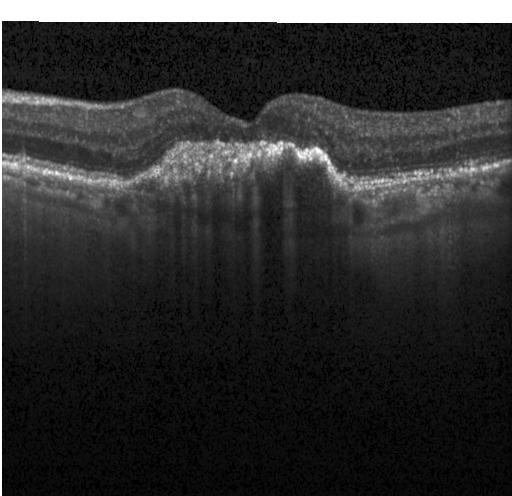 Impression: choroidal neovascularization (CNV).